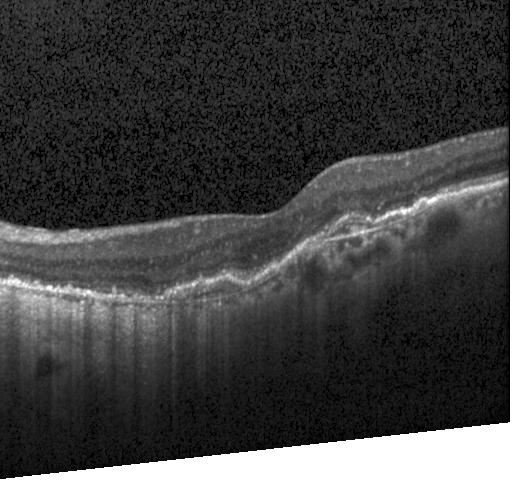

Retinal OCT cross-section · macular scan · Heidelberg Spectralis OCT system
Macular OCT: choroidal neovascularization.